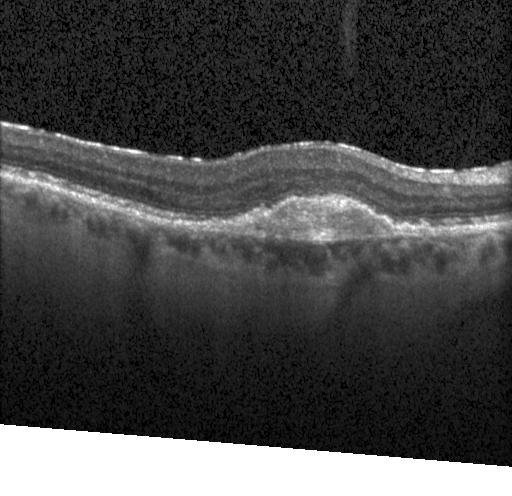
Retinal OCT cross-section
Finding: CNV.